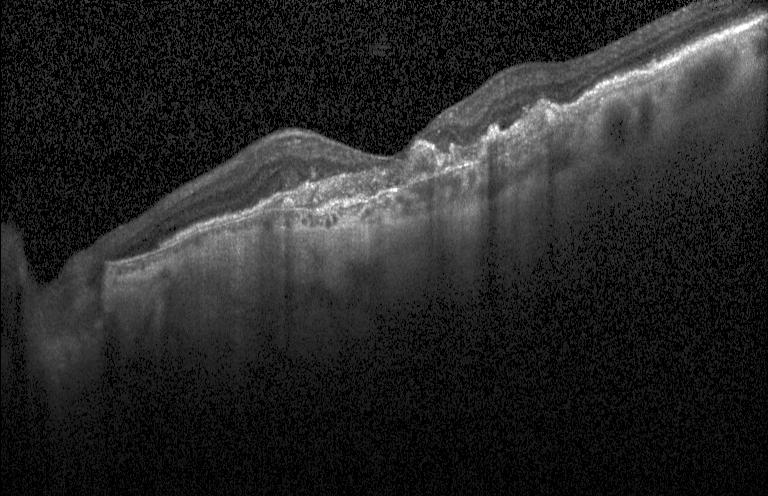 Centered on the fovea, instrument: Heidelberg Spectralis, OCT line scan, spectral-domain OCT.
OCT finding: a choroidal neovascular membrane.